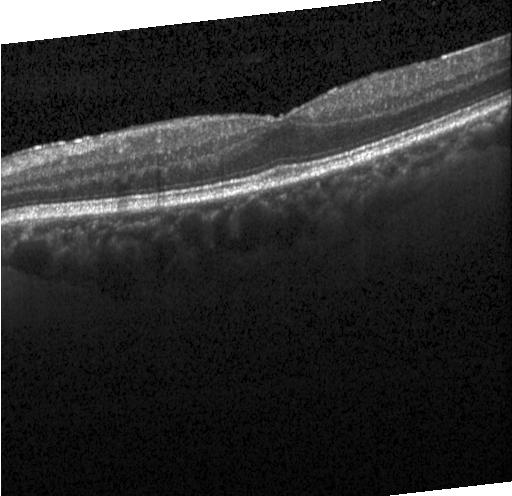
OCT B-scan. Finding: no evidence of choroidal neovascularization, diabetic macular edema, or drusen.